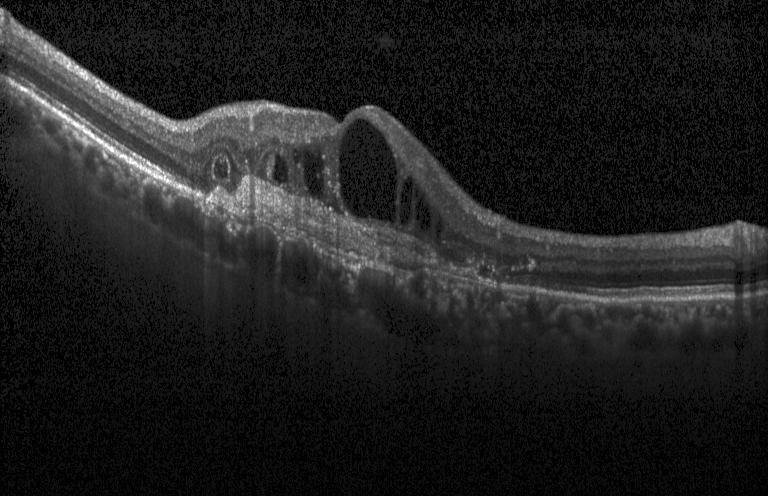 Macular OCT demonstrating a choroidal neovascular membrane.